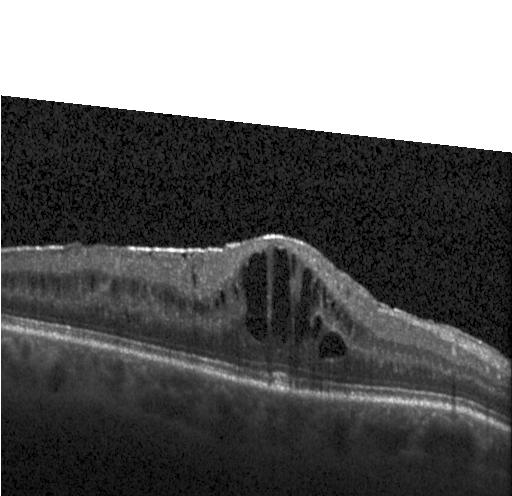 Impression: diabetic macular edema (DME).